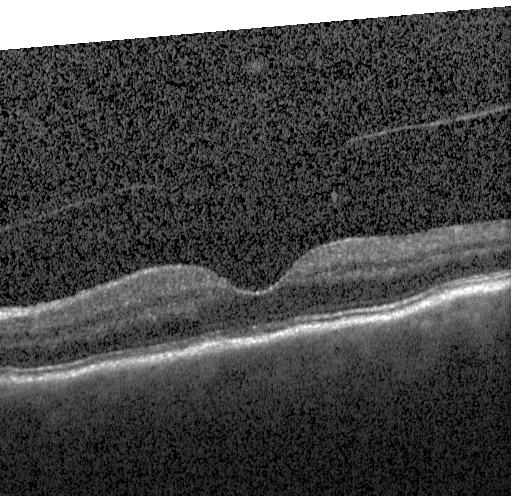

Retinal OCT B-scan. This B-scan demonstrates no choroidal neovascularization, diabetic macular edema, or drusen.